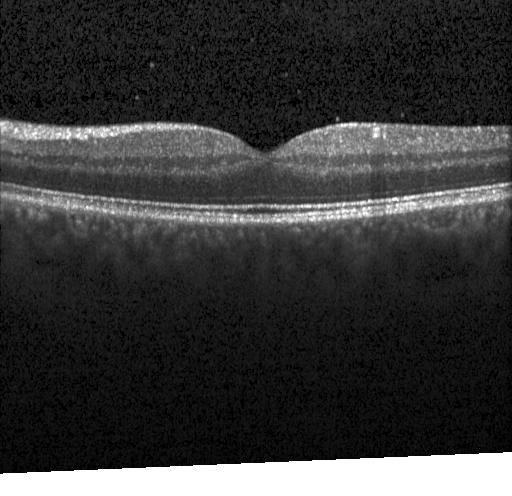

Spectral-domain OCT B-scan: neither choroidal neovascularization, diabetic macular edema, nor drusen.